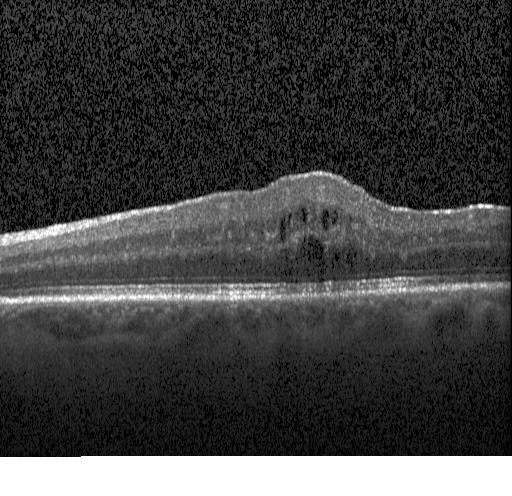
Optical coherence tomography scan. Diagnosis: DME.